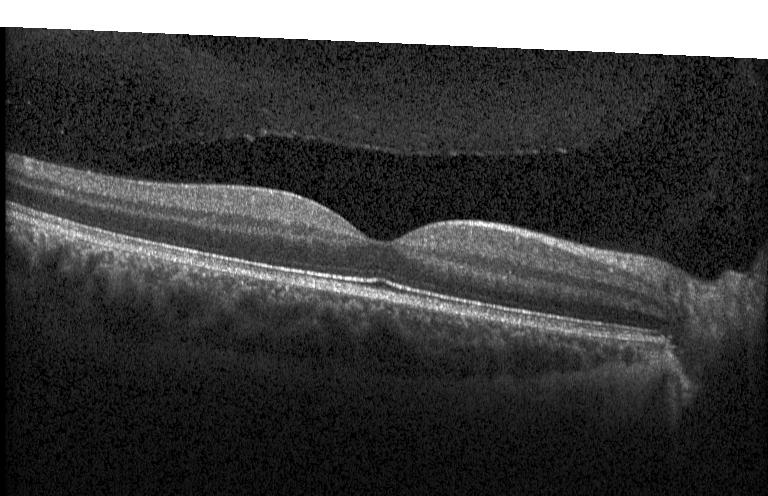

Centered on the fovea; OCT B-scan
Macular OCT: no choroidal neovascularization, no diabetic macular edema, and no drusen.